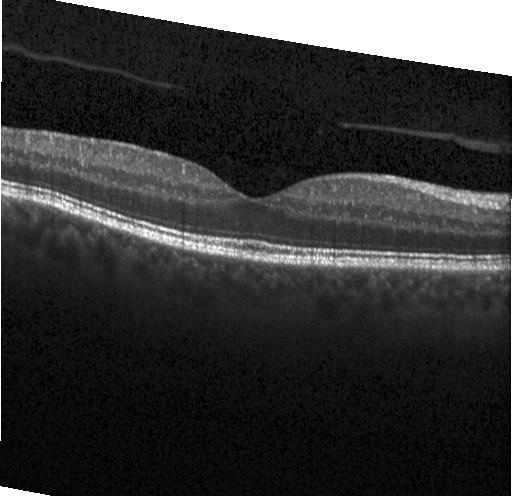
OCT line scan. Diagnosis: no choroidal neovascularization, diabetic macular edema, or drusen.